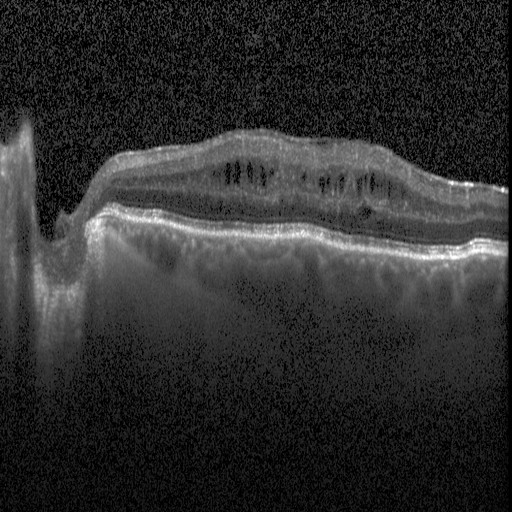

Optical coherence tomography B-scan
Diagnosis: DME.